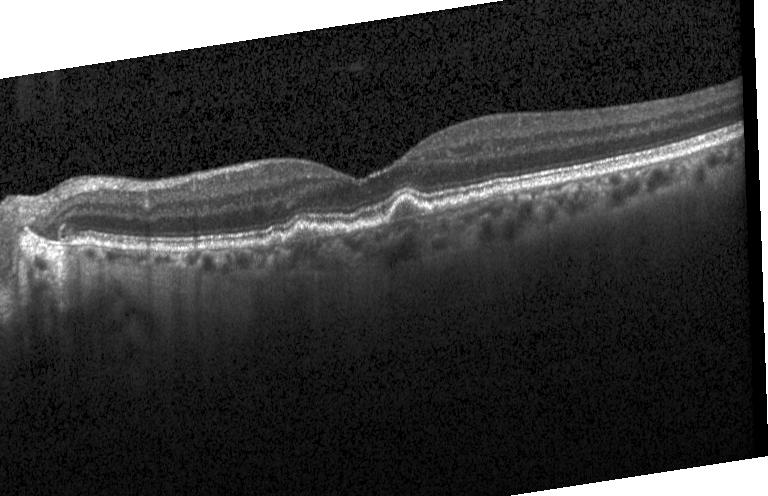

Impression: drusen.